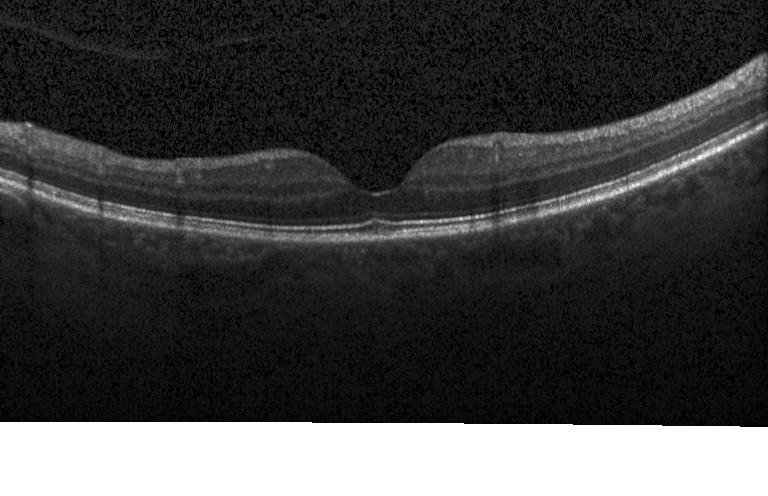

Optical coherence tomography scan
Impression: no choroidal neovascularization, diabetic macular edema, or drusen.